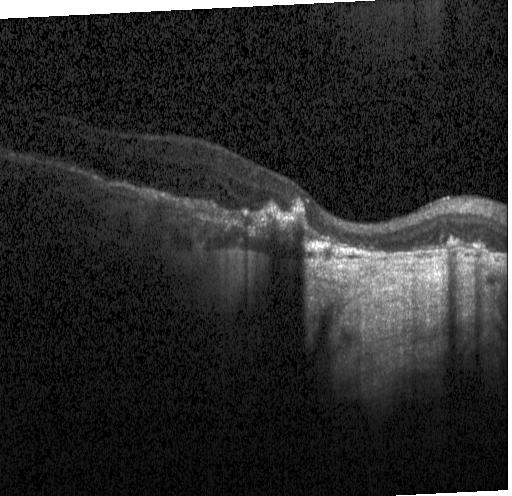

Impression: CNV.